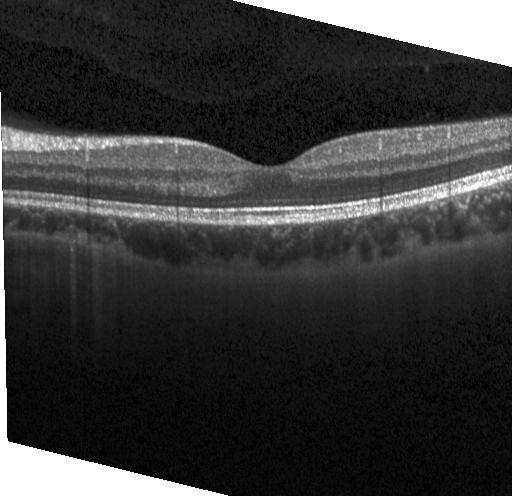

Impression: no evidence of CNV, DME, or drusen.